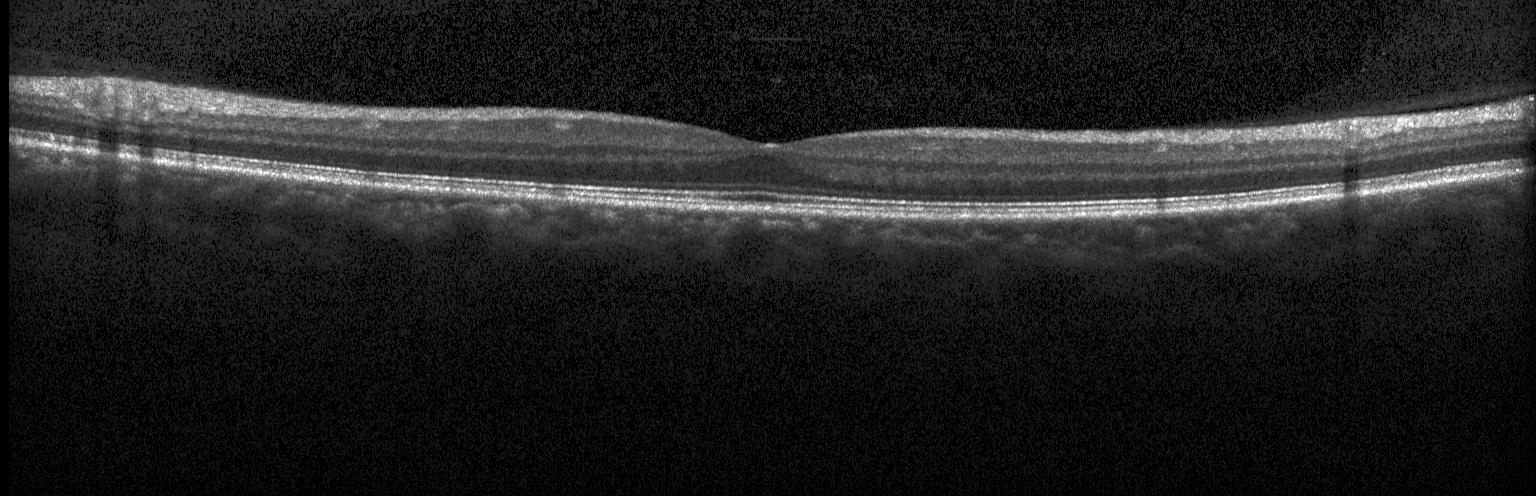

Macular scan; Heidelberg Spectralis; optical coherence tomography B-scan; SD-OCT — Impression: neither CNV, DME, nor drusen.